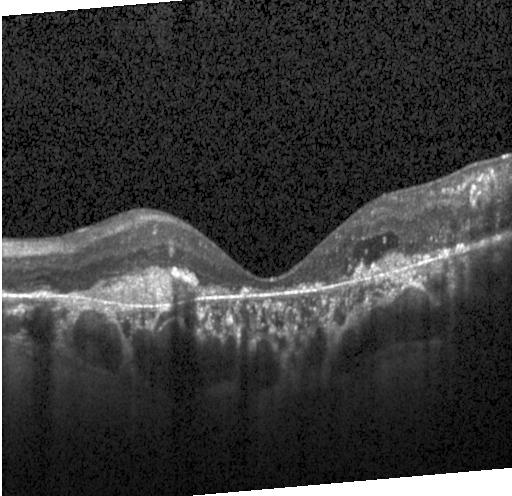

OCT line scan
Macular OCT: a choroidal neovascular membrane.